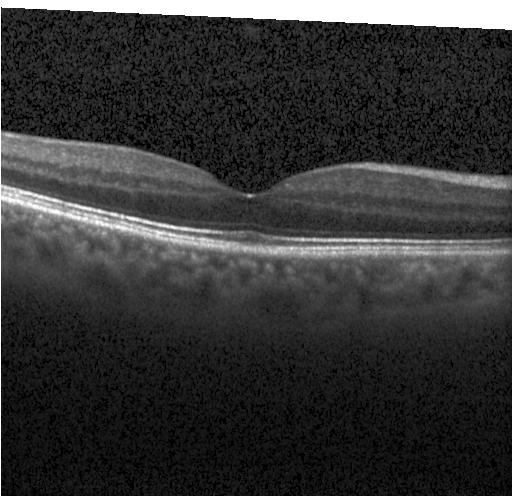 Fovea-centered, optical coherence tomography B-scan — Dx: neither choroidal neovascularization, diabetic macular edema, nor drusen.